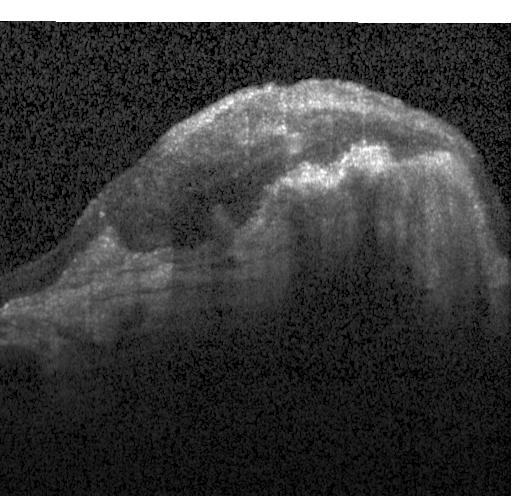
SD-OCT; Heidelberg Spectralis OCT system; centered on the fovea; optical coherence tomography B-scan. Finding: choroidal neovascularization.